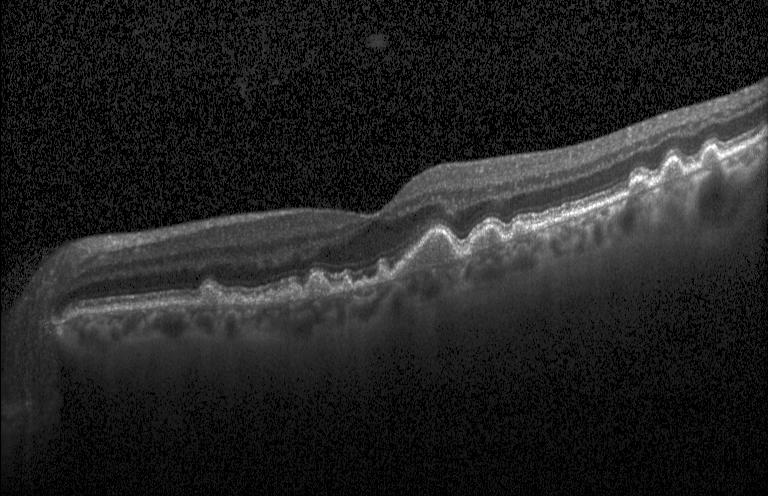 OCT B-scan.
Impression: drusen.